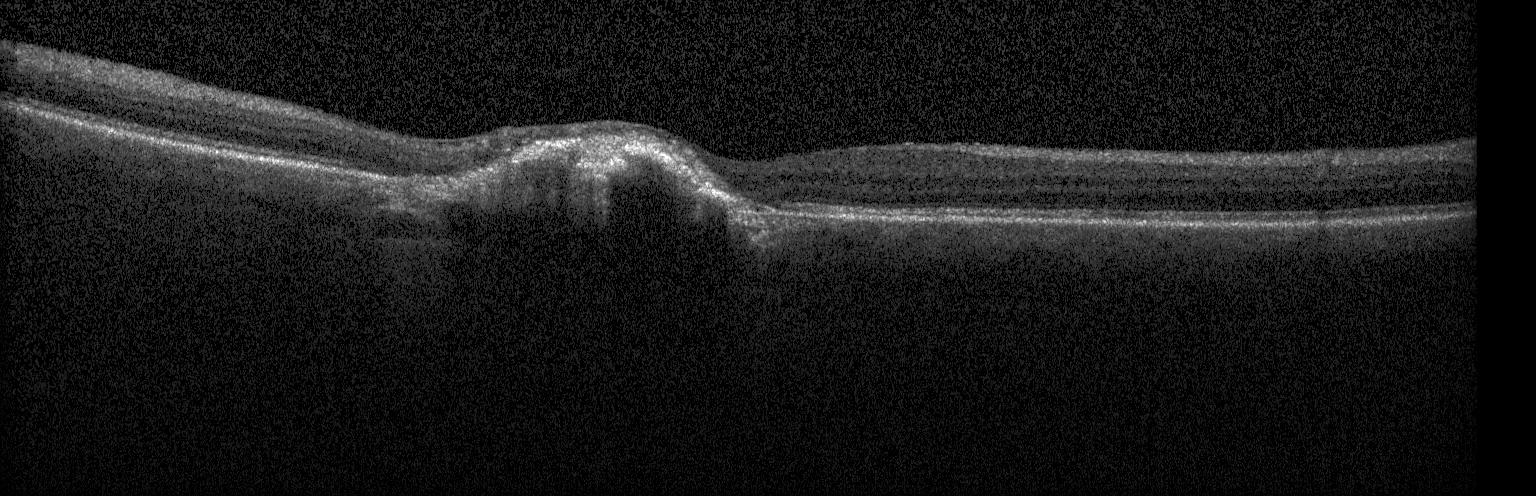

Finding: a choroidal neovascular membrane.